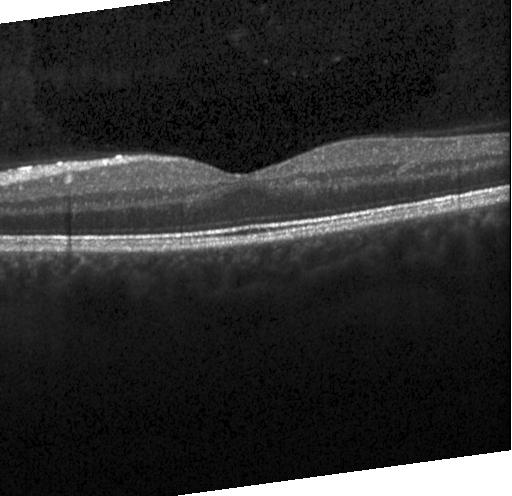

Centered on the fovea, optical coherence tomography B-scan
Assessment: no choroidal neovascularization, no diabetic macular edema, and no drusen.